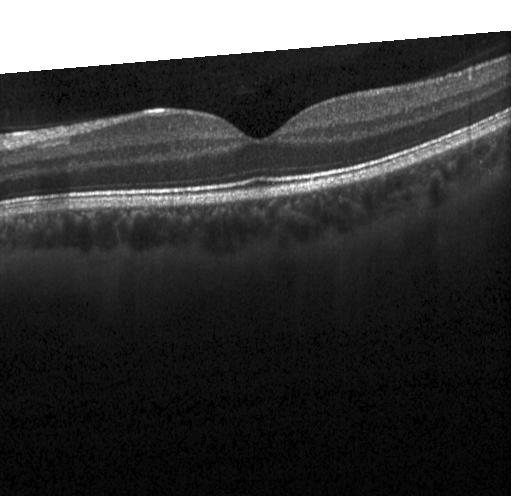 OCT scan showing no choroidal neovascularization, diabetic macular edema, or drusen.